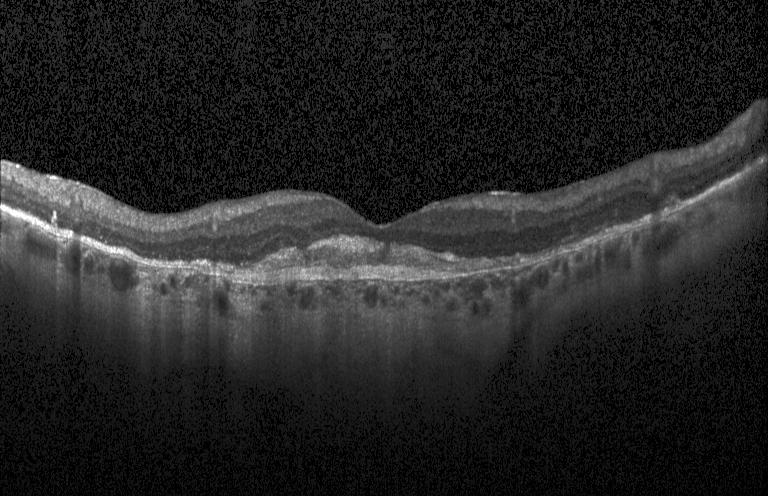

Finding: a choroidal neovascular membrane.